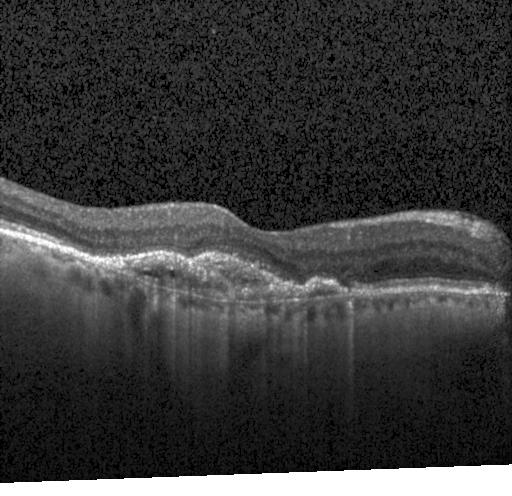
Optical coherence tomography scan.
OCT finding: choroidal neovascularization.